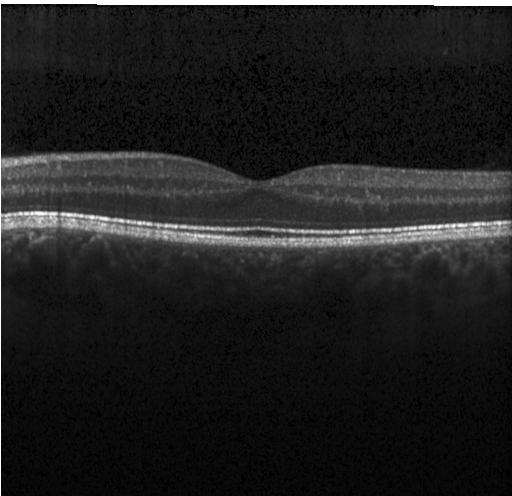

Optical coherence tomography B-scan; spectral-domain optical coherence tomography; horizontal scan through the fovea
Impression: no choroidal neovascularization, diabetic macular edema, or drusen.